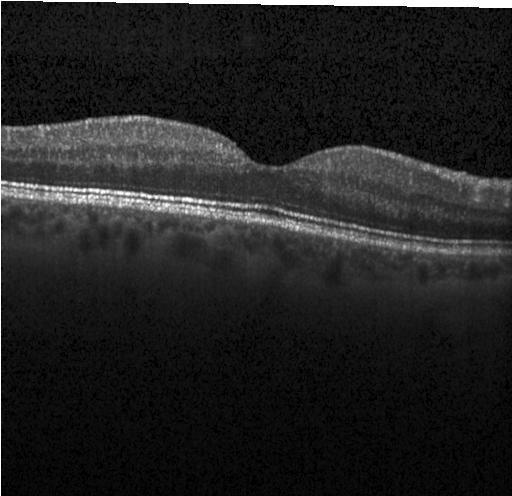
Dx: no choroidal neovascularization, no diabetic macular edema, and no drusen.